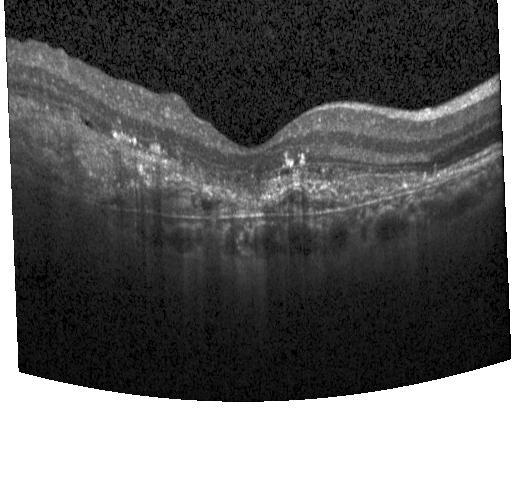

Spectral-domain optical coherence tomography. Retinal OCT cross-section.
Diagnosis: CNV.